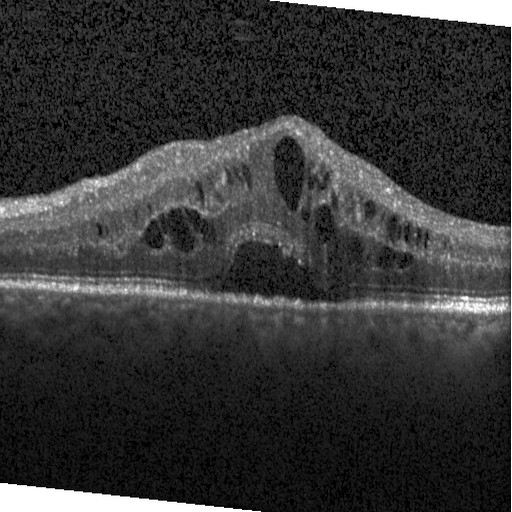
Fovea-centered; Heidelberg Spectralis; OCT B-scan
This B-scan demonstrates diabetic macular edema.